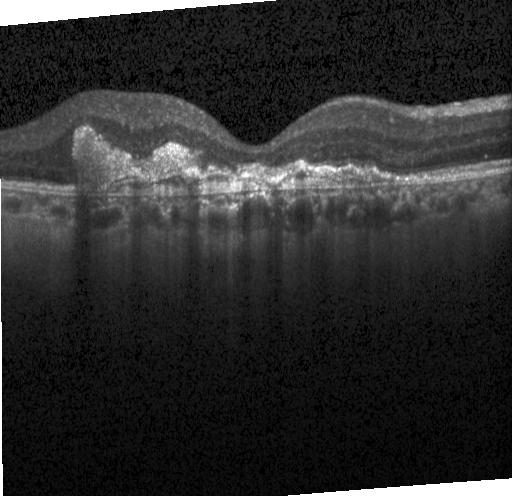
Optical coherence tomography scan; Heidelberg Spectralis; fovea-centered — OCT finding: a choroidal neovascular membrane.